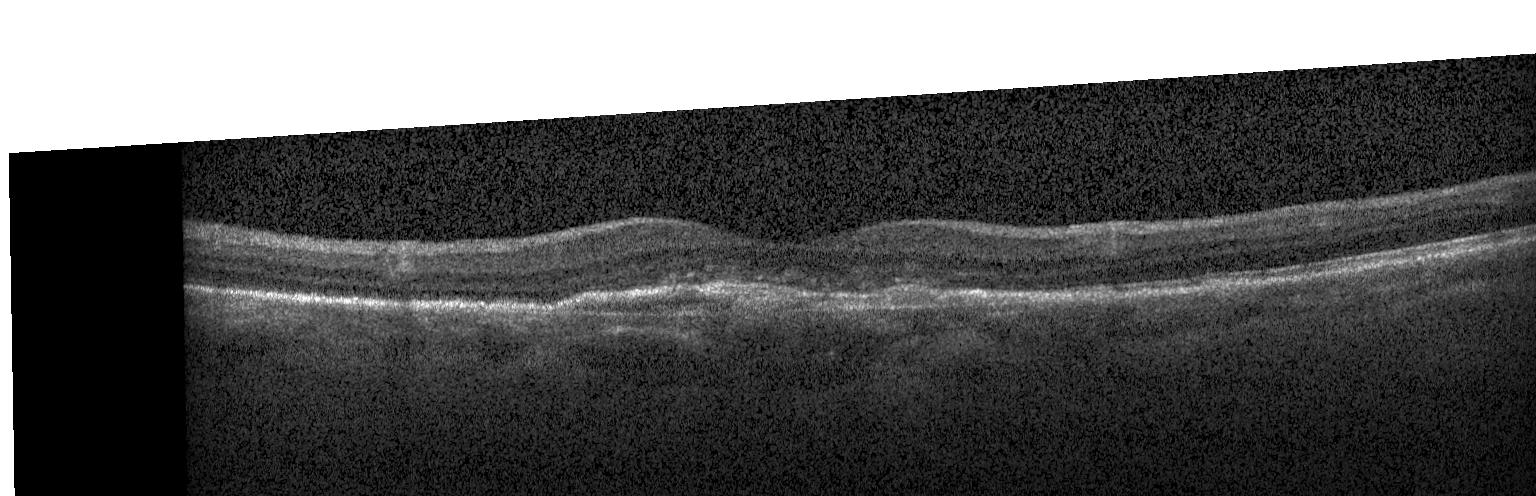 OCT B-scan
OCT finding: choroidal neovascularization.